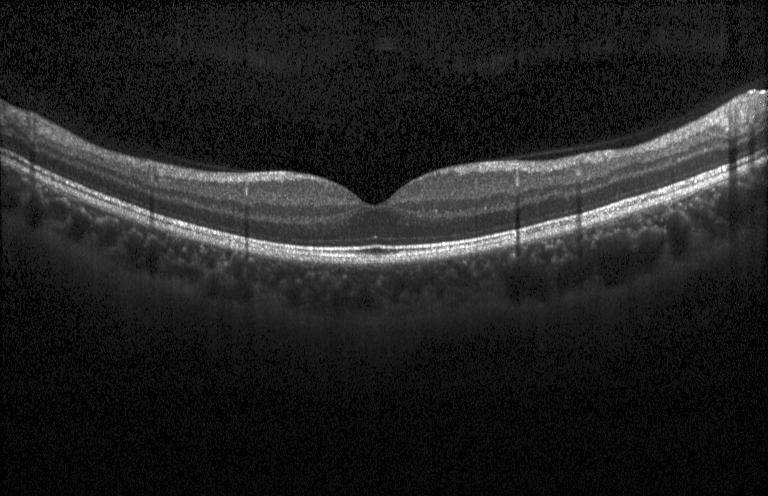
Retinal OCT cross-section — OCT finding: neither choroidal neovascularization, diabetic macular edema, nor drusen.